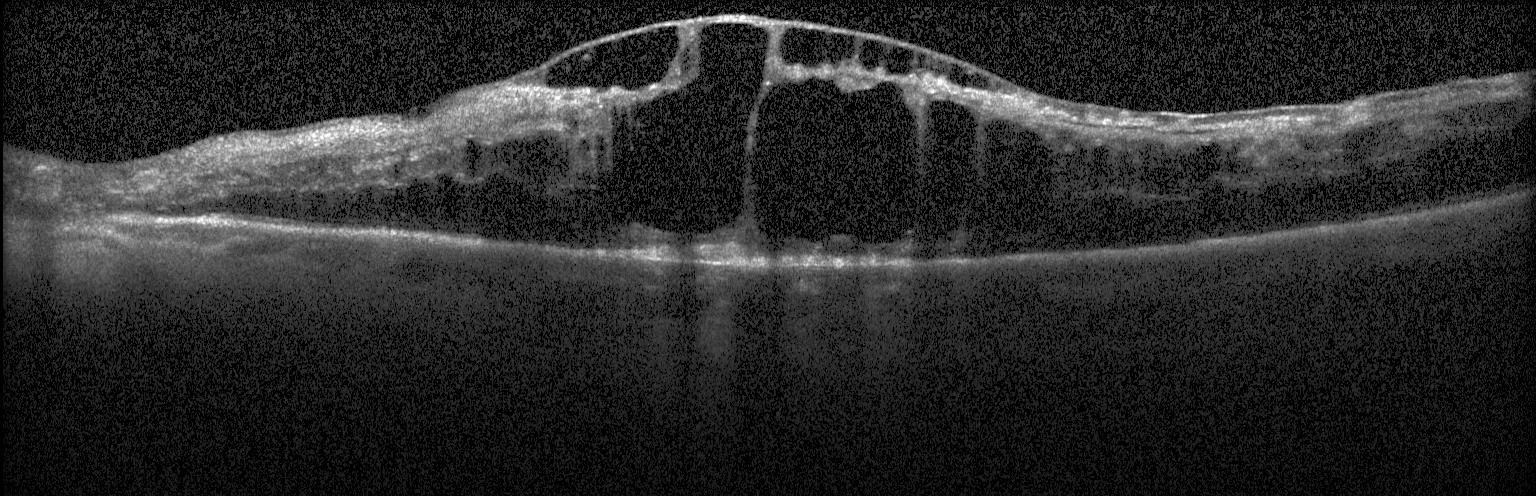

Spectral-domain OCT B-scan: DME.